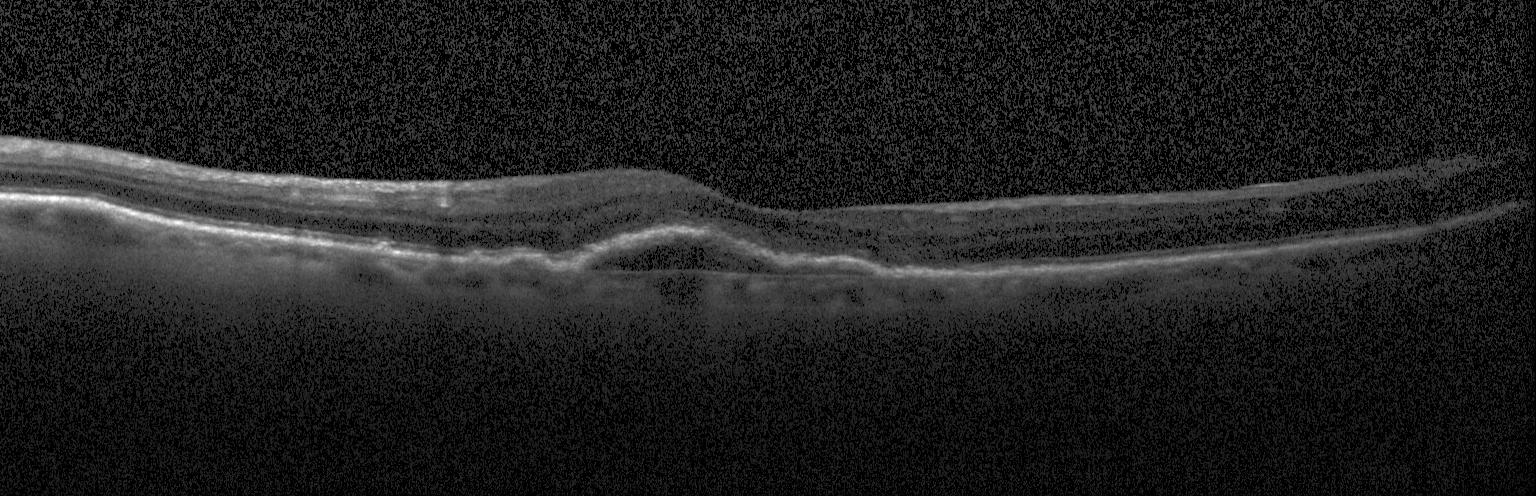 Optical coherence tomography B-scan · SD-OCT · instrument: Heidelberg Spectralis. Impression: a choroidal neovascular membrane.